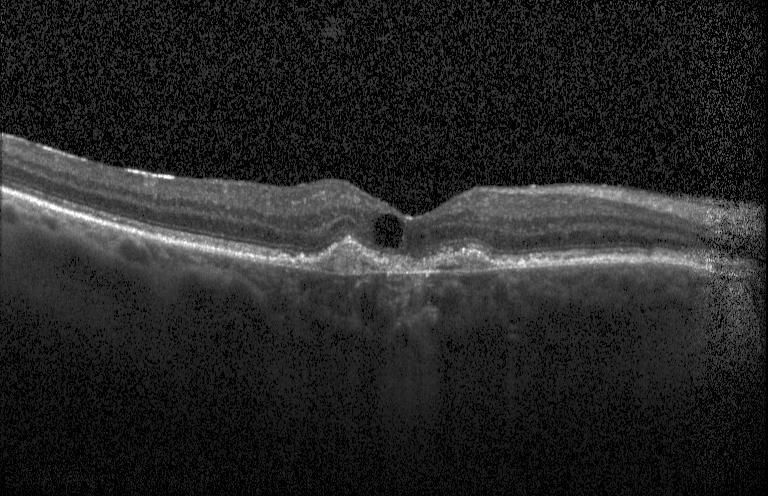

OCT B-scan · acquired on a Heidelberg Spectralis — This B-scan demonstrates choroidal neovascularization (CNV).